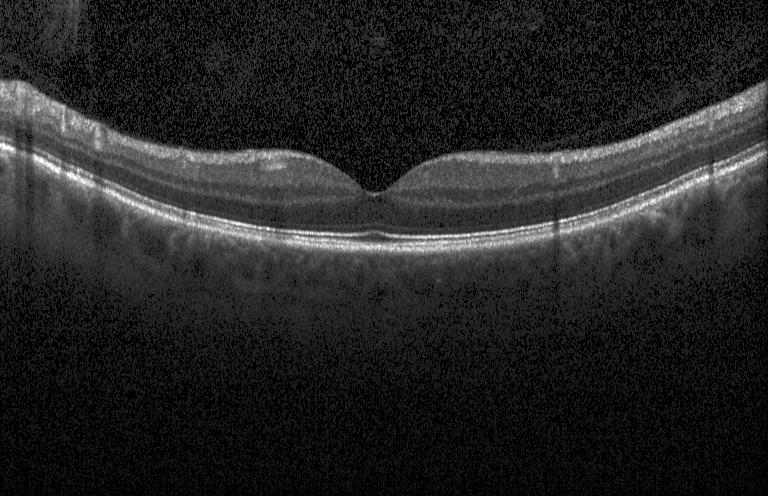 Diagnosis: neither CNV, DME, nor drusen.